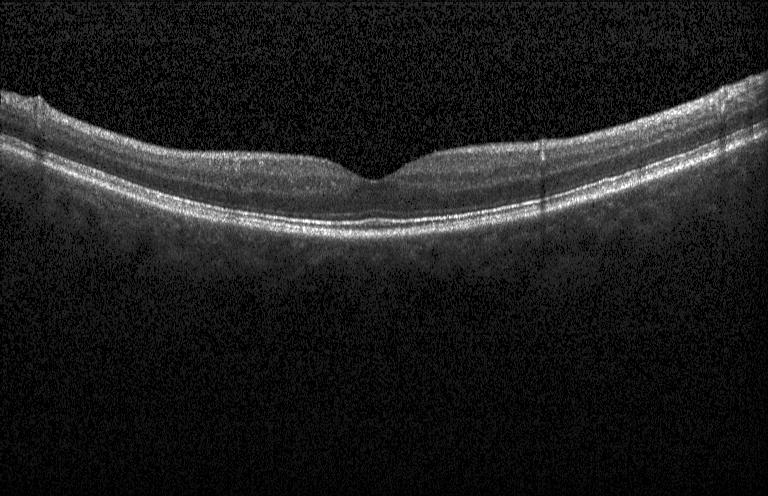
Retinal OCT cross-section — Assessment: neither choroidal neovascularization, diabetic macular edema, nor drusen.